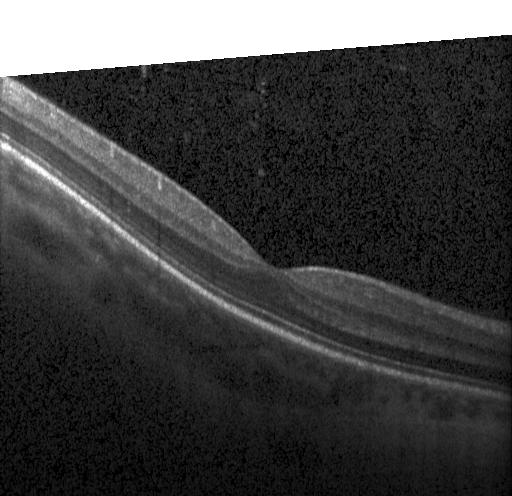 Centered on the fovea; OCT line scan; spectral-domain OCT; Heidelberg Spectralis.
Macular OCT: no evidence of choroidal neovascularization, diabetic macular edema, or drusen.